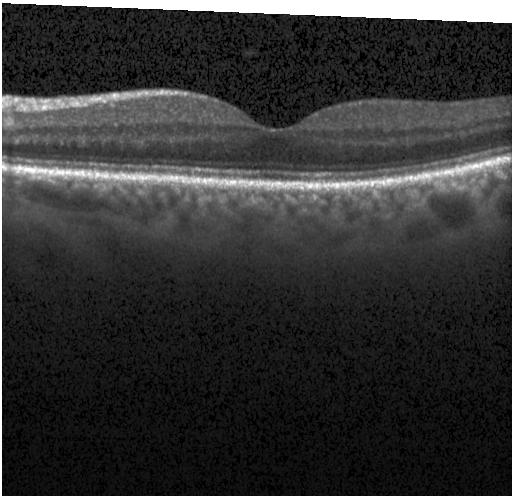
Macular OCT demonstrating no choroidal neovascularization, no diabetic macular edema, and no drusen.